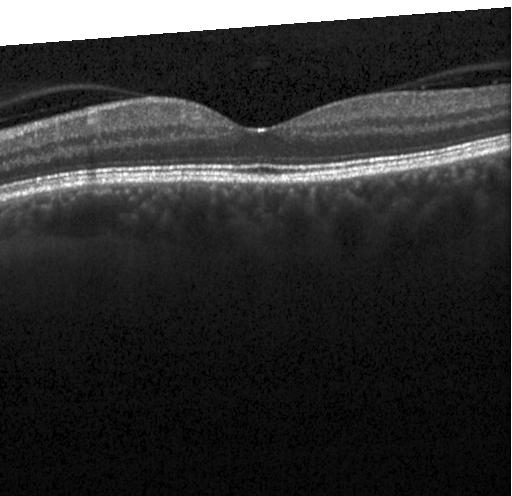 Retinal OCT cross-section — Finding: no evidence of CNV, DME, or drusen.